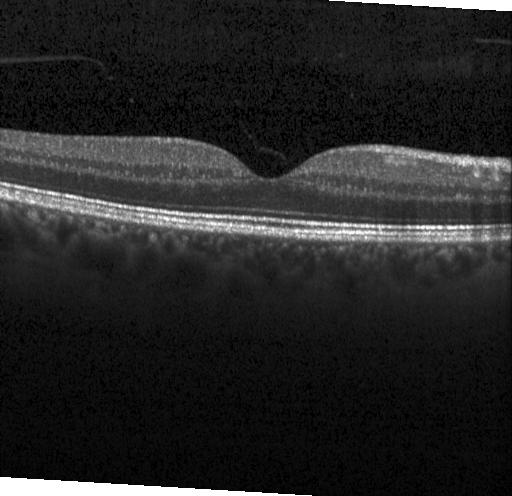

Optical coherence tomography B-scan; Heidelberg Spectralis; spectral-domain optical coherence tomography; through the macula.
Diagnosis: no evidence of CNV, DME, or drusen.